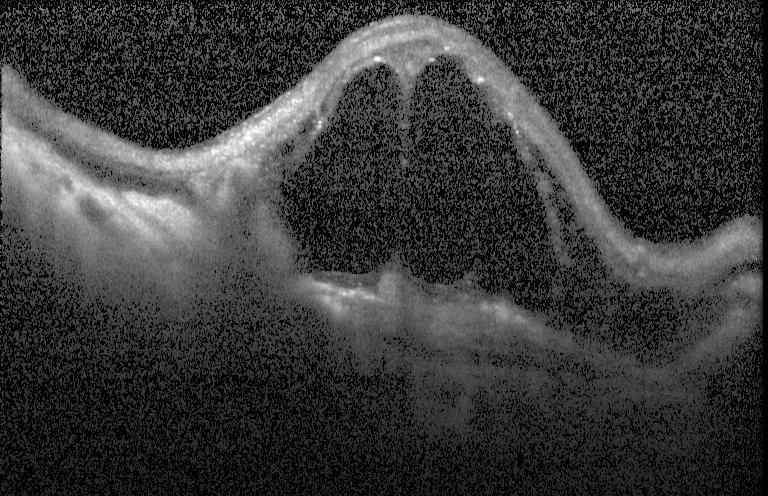
Dx: DME.